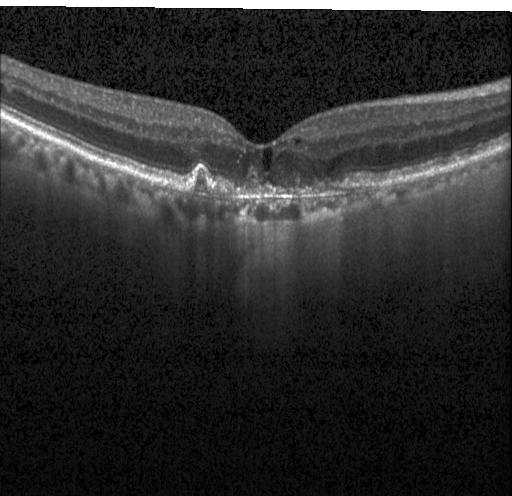 Retinal OCT cross-section showing choroidal neovascularization.